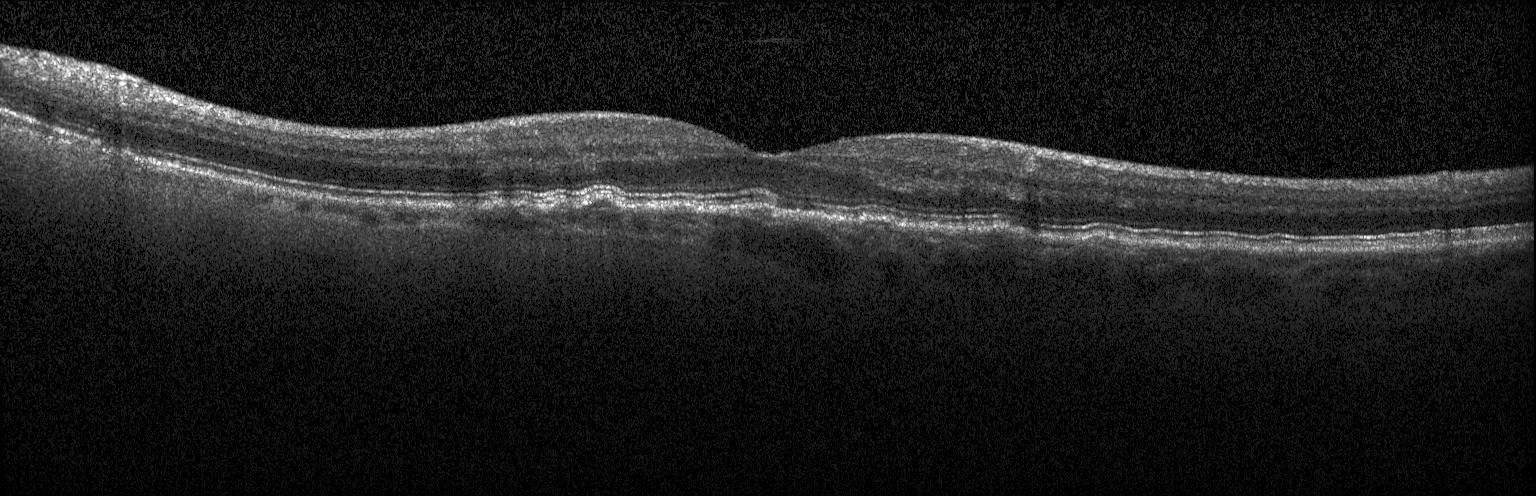

Macular OCT demonstrating drusen.